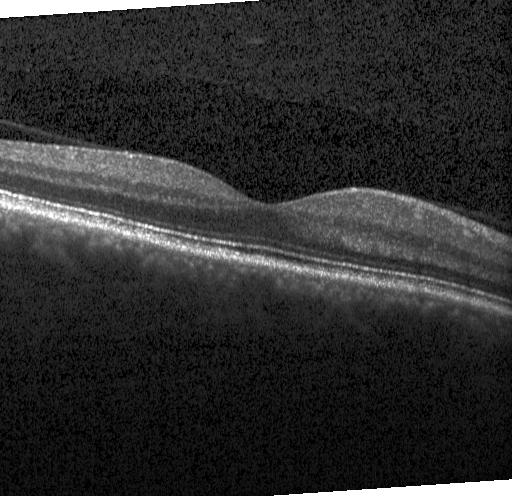
Dx: no evidence of choroidal neovascularization, diabetic macular edema, or drusen.